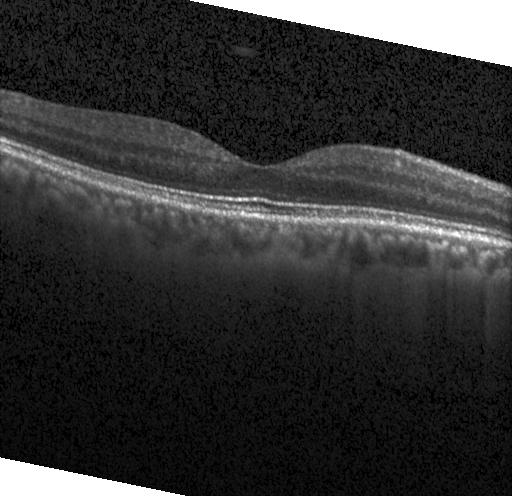 OCT finding: no choroidal neovascularization, diabetic macular edema, or drusen.